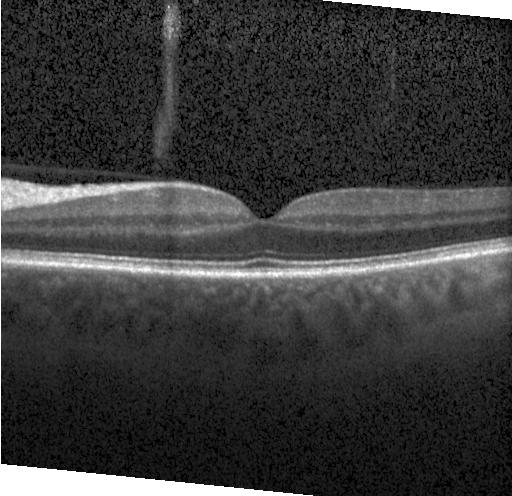
Optical coherence tomography scan. No evidence of CNV, DME, or drusen.